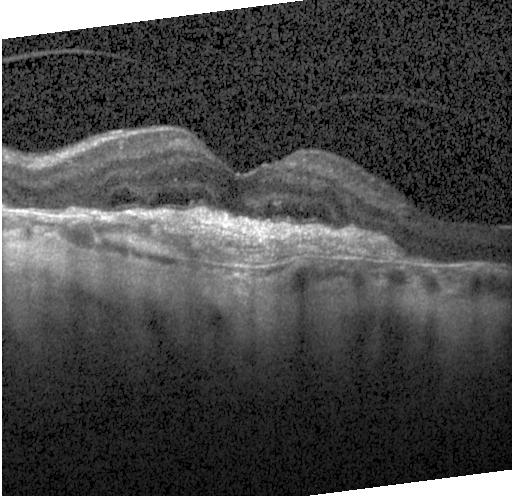
Centered on the fovea. Optical coherence tomography scan. Spectral-domain OCT. Instrument: Heidelberg Spectralis — Impression: CNV.